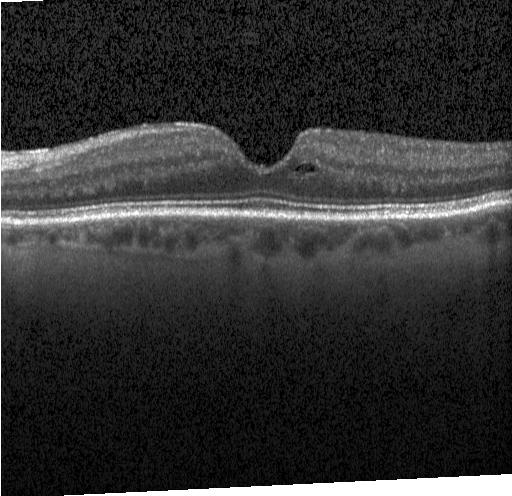
Optical coherence tomography scan. Finding: diabetic macular edema (DME).